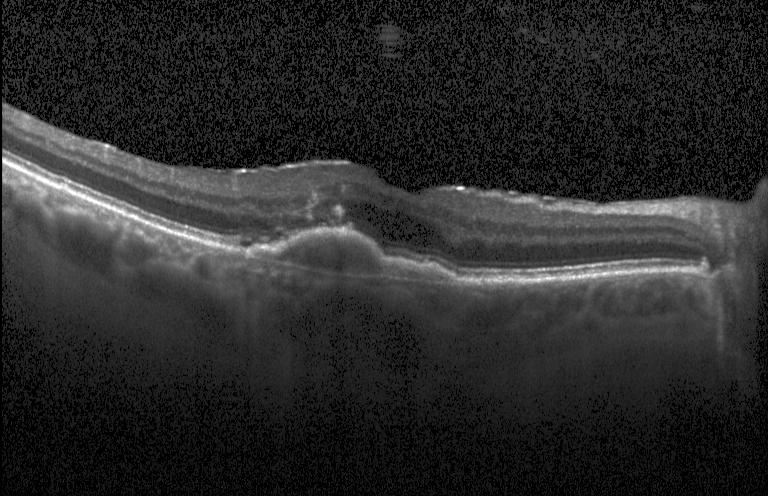
Instrument: Heidelberg Spectralis, OCT B-scan, horizontal scan through the fovea, spectral-domain OCT. Diagnosis: a choroidal neovascular membrane.